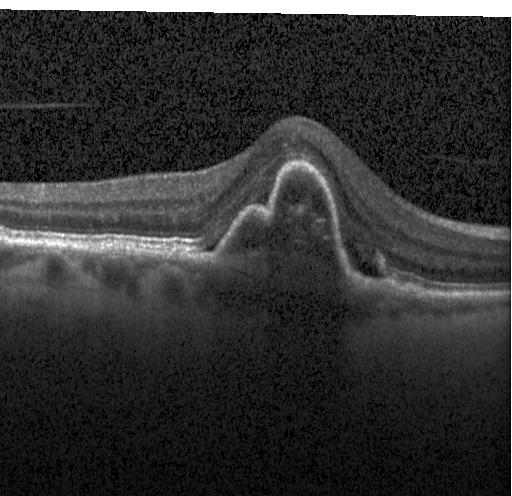 Finding: a choroidal neovascular membrane.